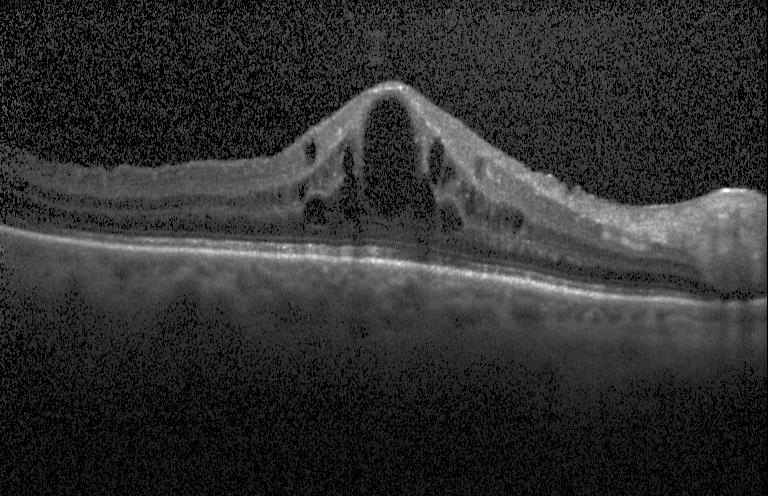
Acquired on a Heidelberg Spectralis. OCT line scan. Horizontal scan through the fovea.
This B-scan demonstrates DME.